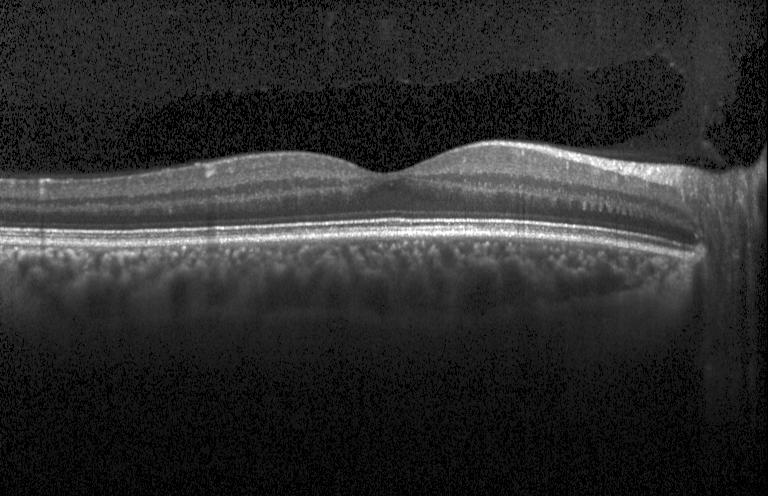

Dx: no choroidal neovascularization, no diabetic macular edema, and no drusen.